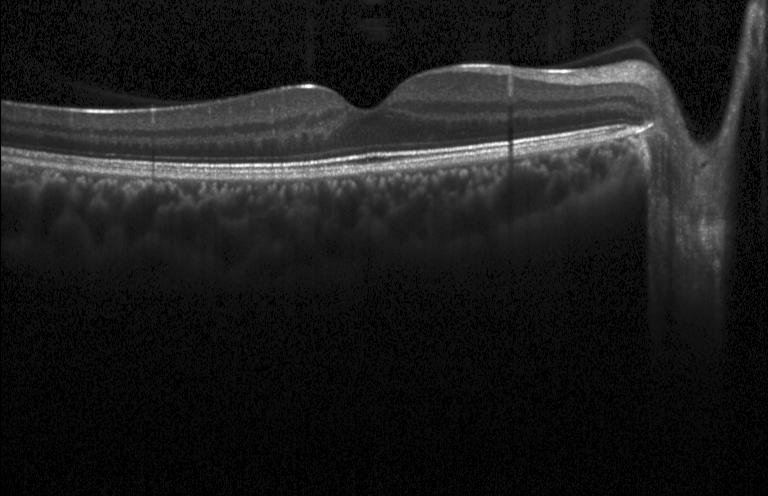 Retinal OCT cross-section showing no CNV, DME, or drusen.